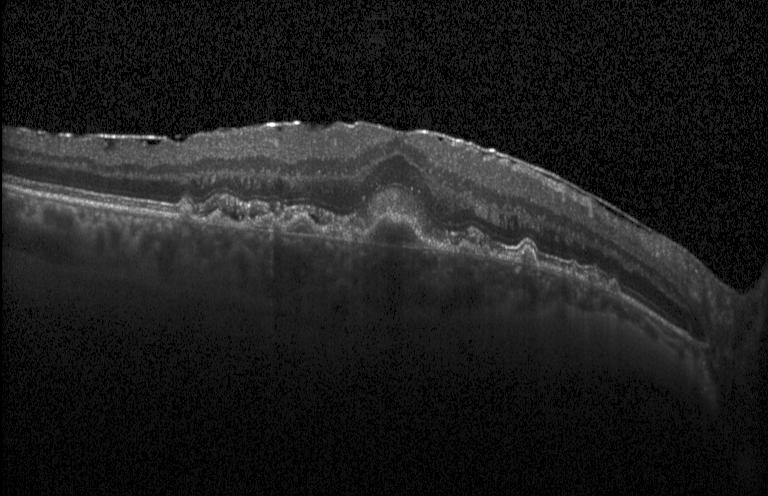
OCT B-scan showing a choroidal neovascular membrane.